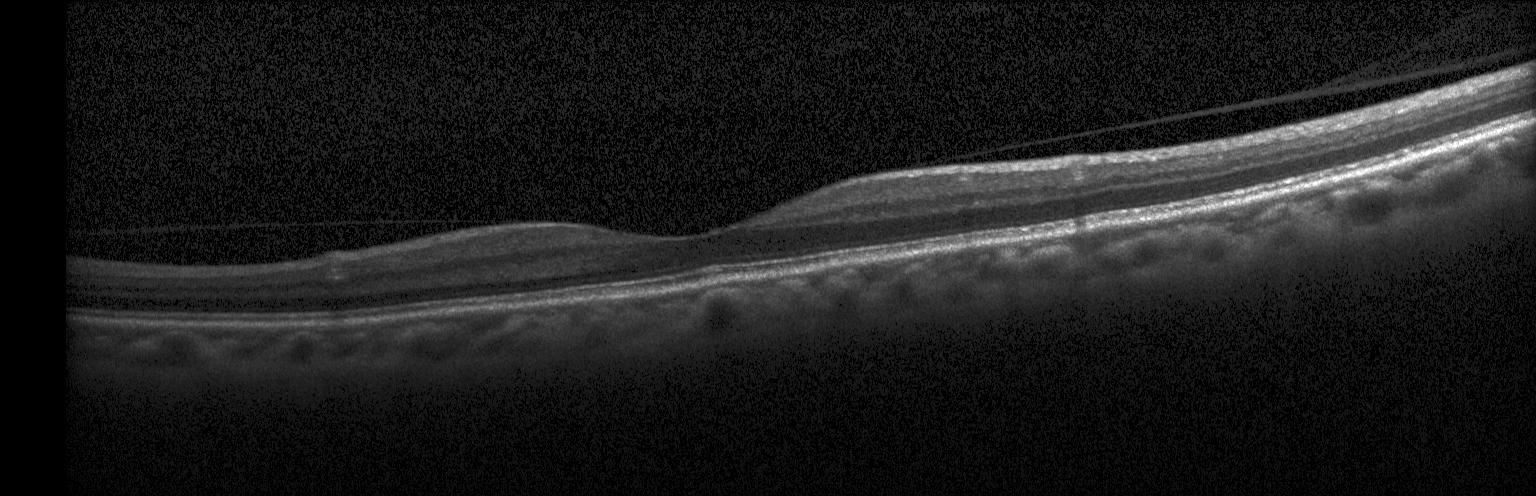 OCT line scan; macular scan
Diagnosis: no choroidal neovascularization, no diabetic macular edema, and no drusen.